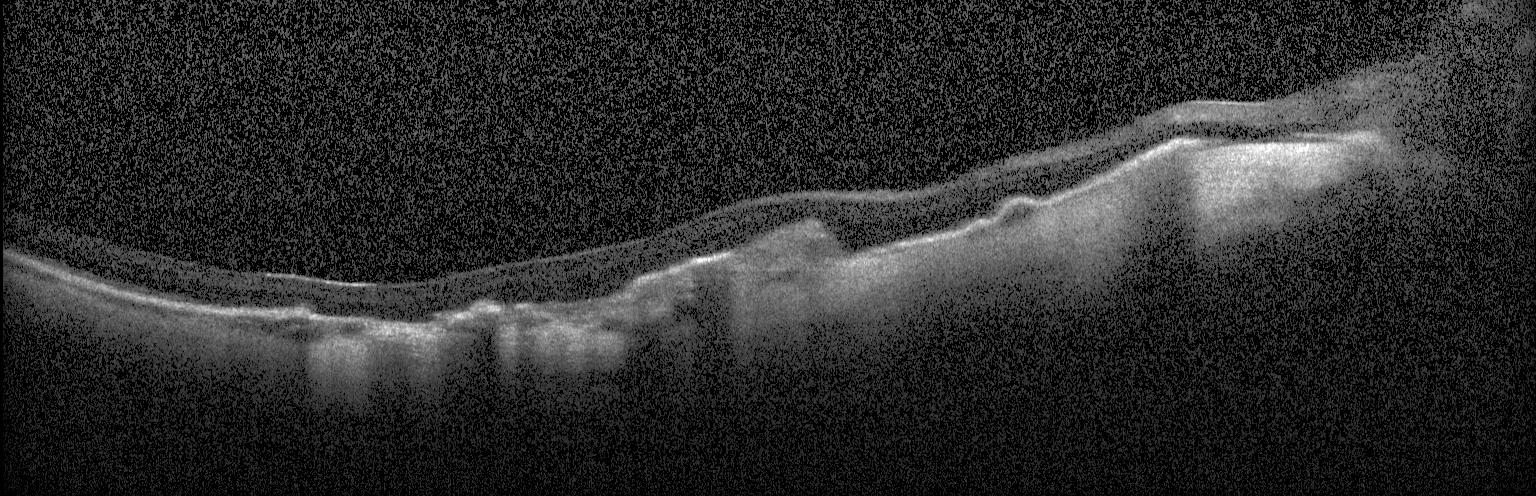

Optical coherence tomography scan, spectral-domain optical coherence tomography
The scan shows choroidal neovascularization.